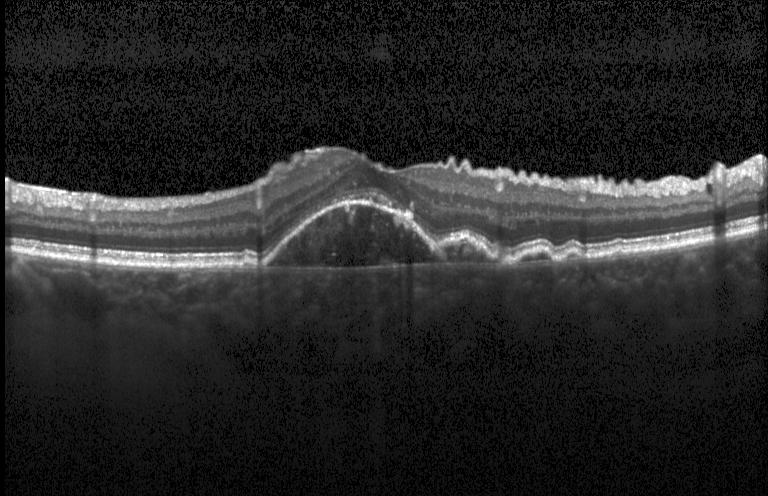 Diagnosis: choroidal neovascularization.